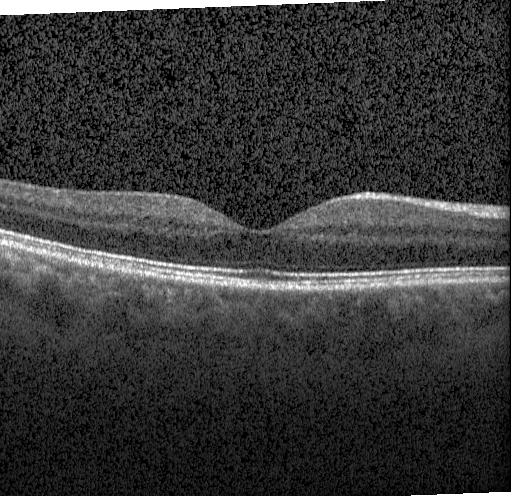 Retinal OCT B-scan.
Impression: no evidence of CNV, DME, or drusen.